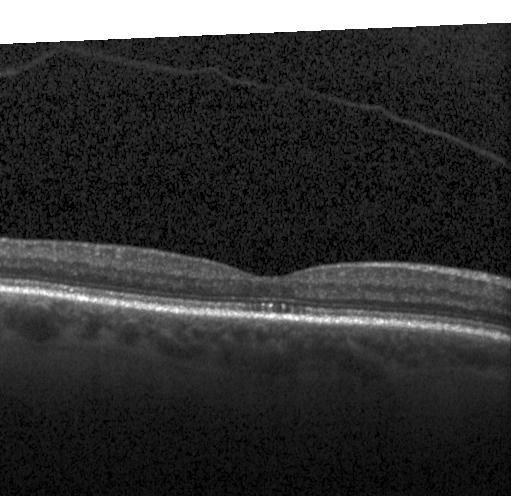

Heidelberg Spectralis OCT system. Horizontal scan through the fovea. Spectral-domain OCT. Retinal OCT cross-section. Impression: no choroidal neovascularization, no diabetic macular edema, and no drusen.